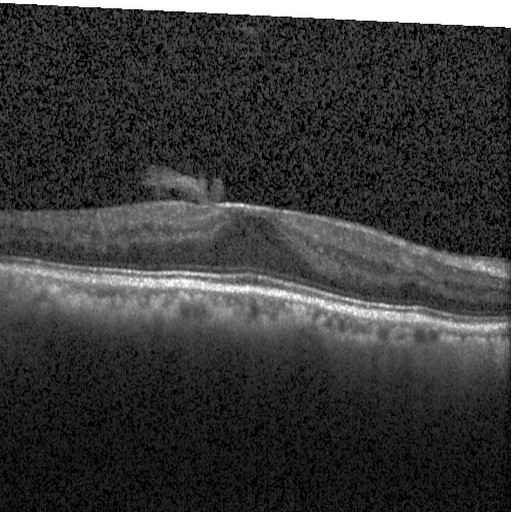
OCT scan showing diabetic macular edema.